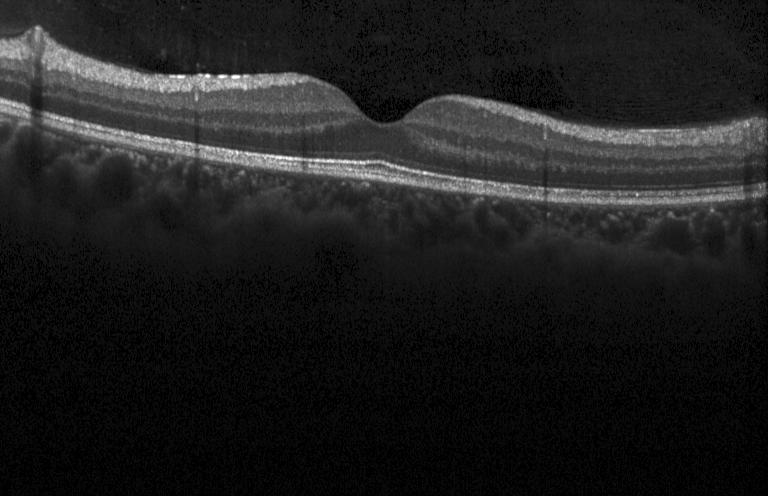 Spectral-domain OCT. OCT line scan.
Finding: no evidence of CNV, DME, or drusen.